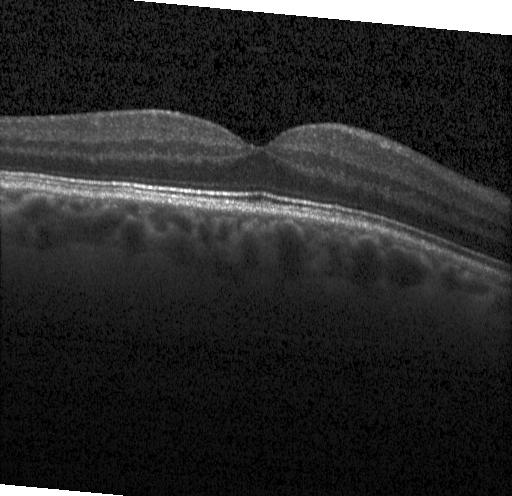
OCT B-scan.
Finding: no choroidal neovascularization, diabetic macular edema, or drusen.